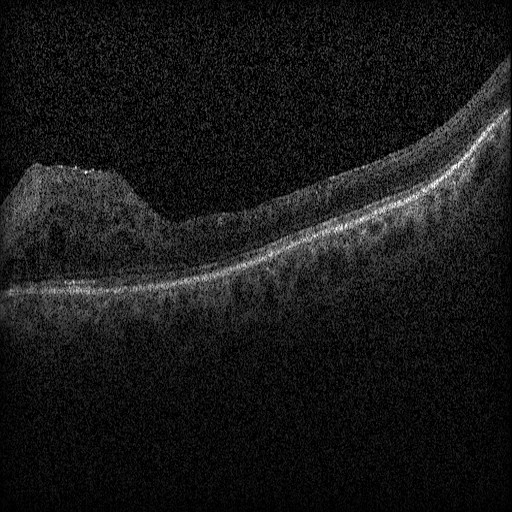
Heidelberg Spectralis, horizontal scan through the fovea, retinal OCT B-scan. OCT finding: DME.